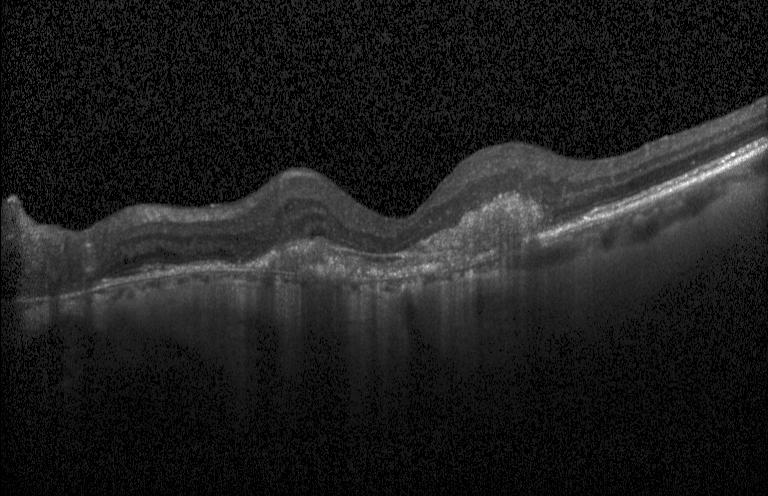
A choroidal neovascular membrane.